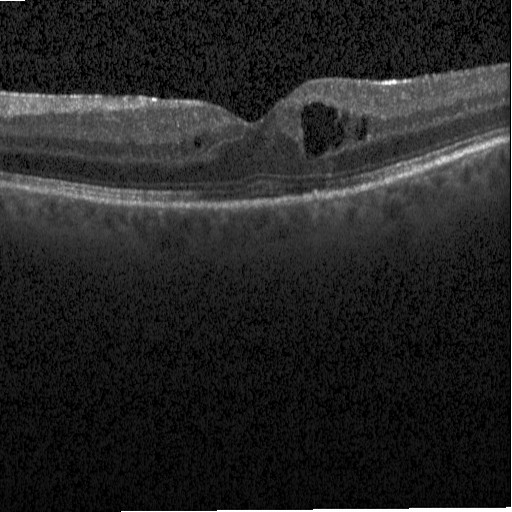

Retinal OCT B-scan. Assessment: diabetic macular edema.